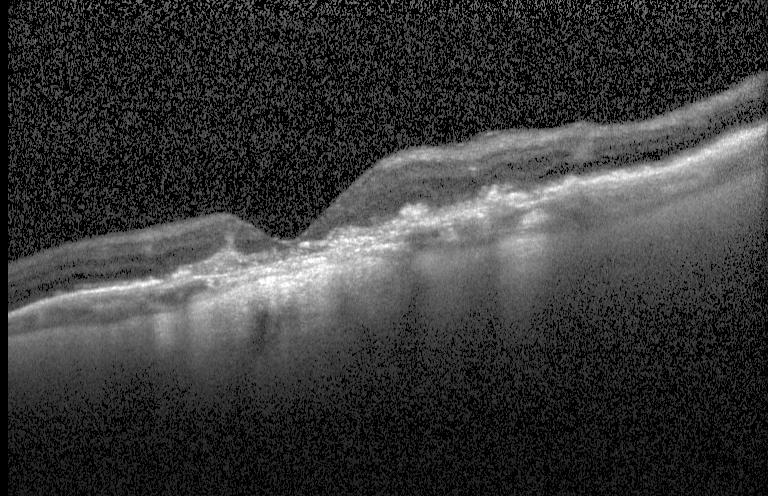

A choroidal neovascular membrane.